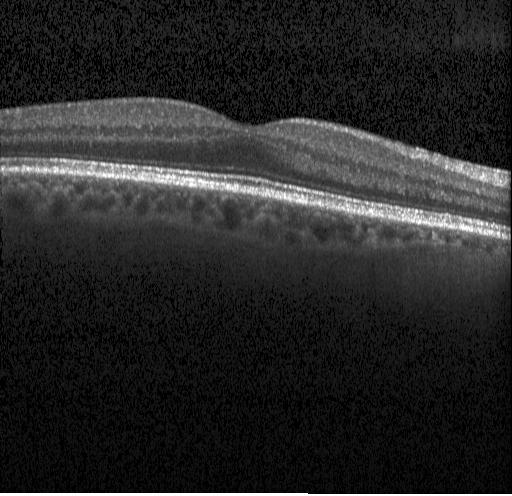
SD-OCT. Optical coherence tomography scan. Heidelberg Spectralis OCT system — Finding: no choroidal neovascularization, no diabetic macular edema, and no drusen.